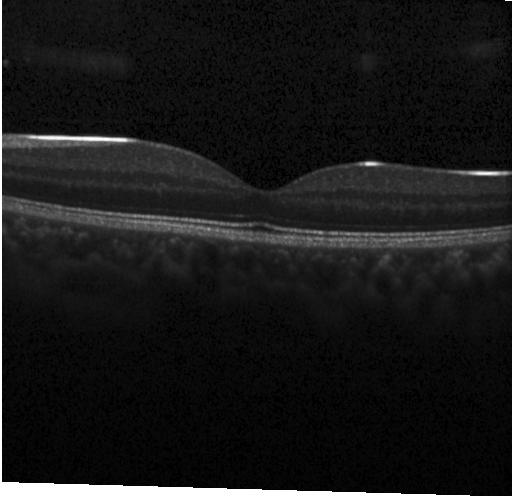

Centered on the fovea. Instrument: Heidelberg Spectralis. OCT B-scan. Spectral-domain OCT — OCT finding: no evidence of choroidal neovascularization, diabetic macular edema, or drusen.